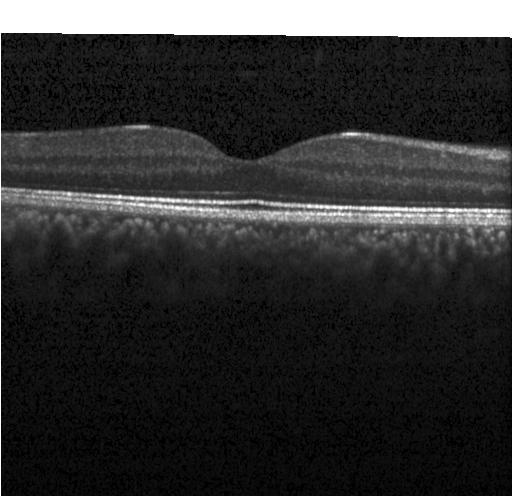 Fovea-centered. Heidelberg Spectralis. Optical coherence tomography B-scan. Spectral-domain OCT
This B-scan demonstrates no evidence of choroidal neovascularization, diabetic macular edema, or drusen.